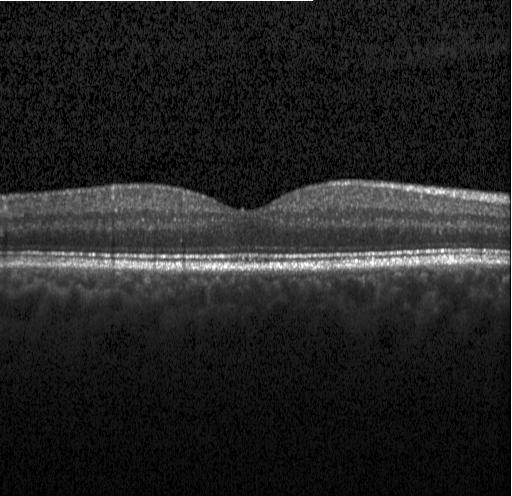 Retinal OCT B-scan. Neither CNV, DME, nor drusen.